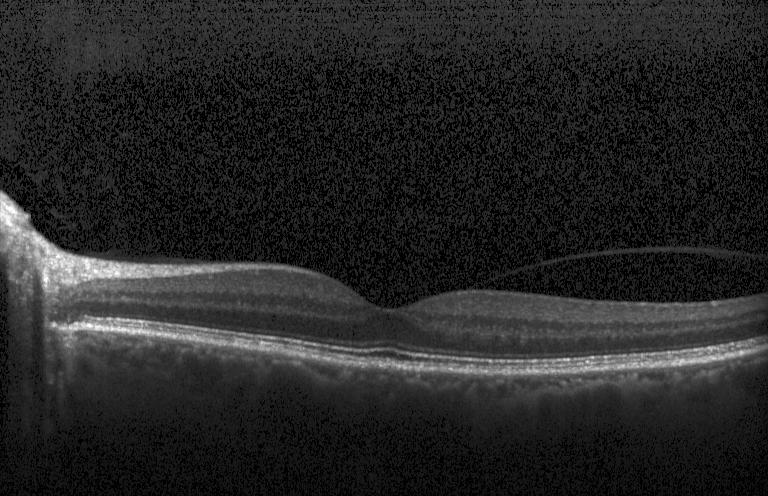

Optical coherence tomography B-scan. Macular scan — Finding: no CNV, DME, or drusen.